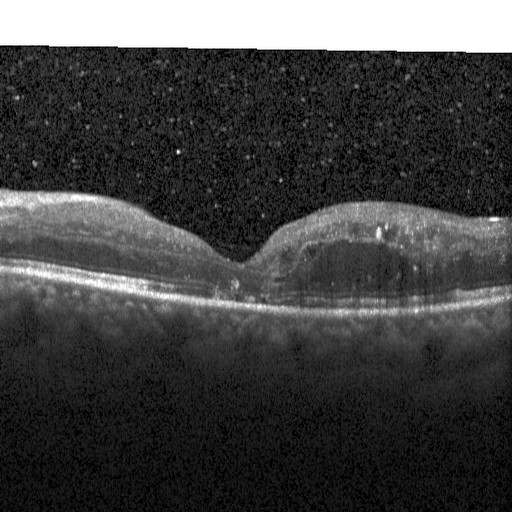
OCT line scan, spectral-domain optical coherence tomography
Diabetic macular edema.